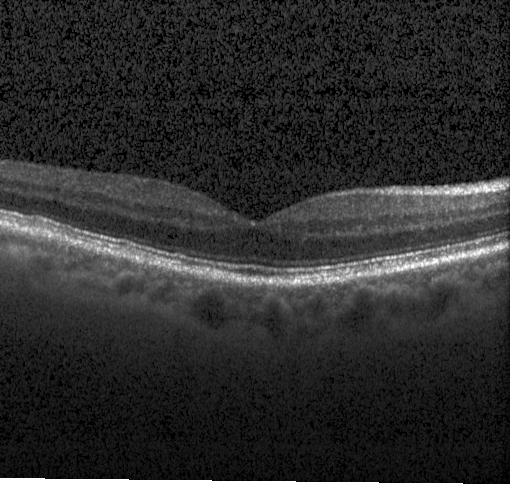
Spectral-domain OCT B-scan: no CNV, no DME, and no drusen.